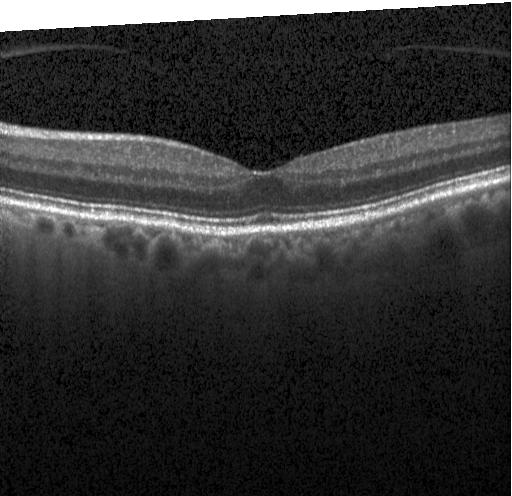
Retinal OCT cross-section. Acquired on a Heidelberg Spectralis. Assessment: no CNV, no DME, and no drusen.